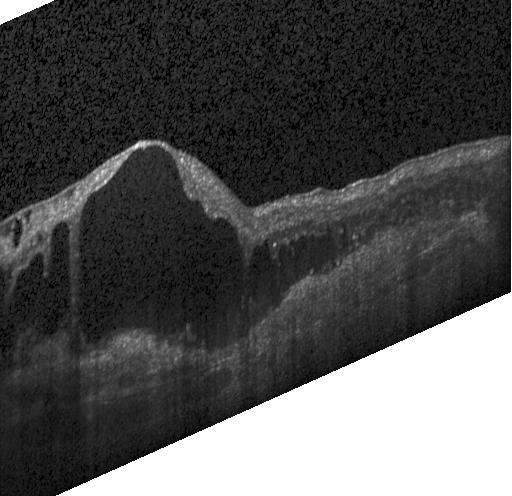

OCT finding: choroidal neovascularization.